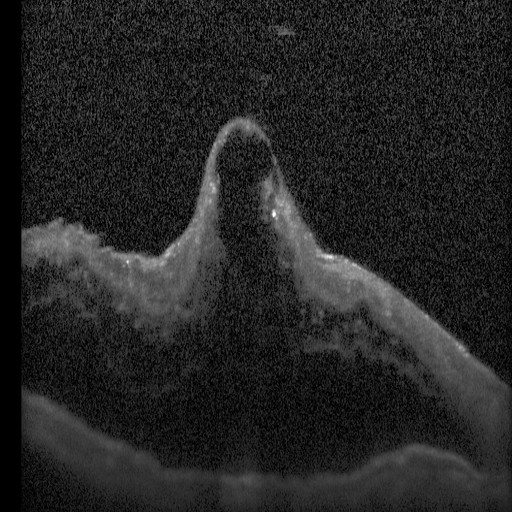
OCT line scan. Heidelberg Spectralis OCT system — Diabetic macular edema.